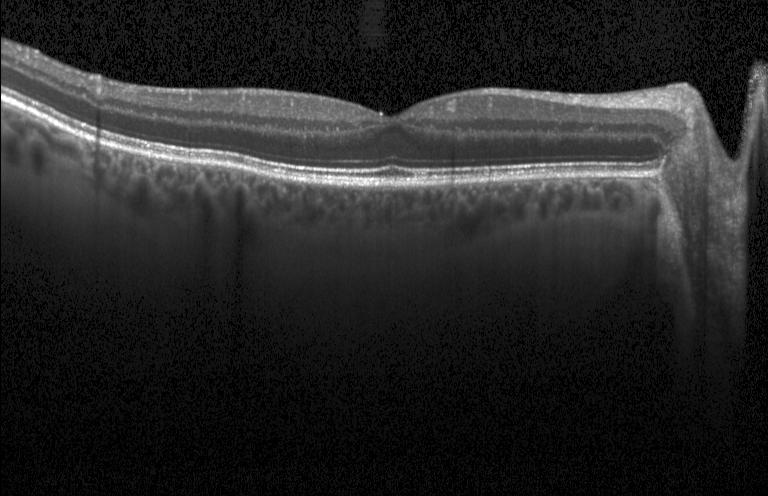

Acquired on a Heidelberg Spectralis; OCT line scan; SD-OCT
Diagnosis: no choroidal neovascularization, diabetic macular edema, or drusen.